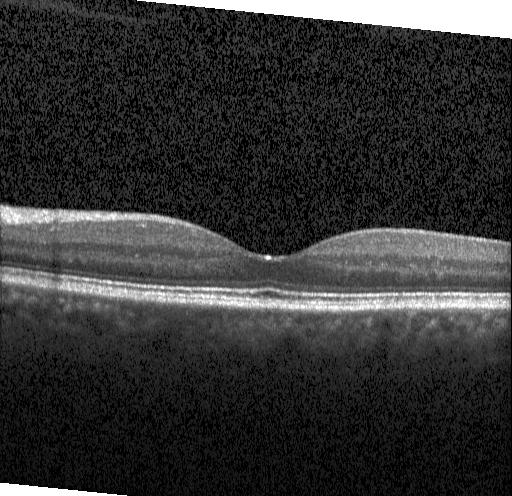
Diagnosis: no evidence of choroidal neovascularization, diabetic macular edema, or drusen.